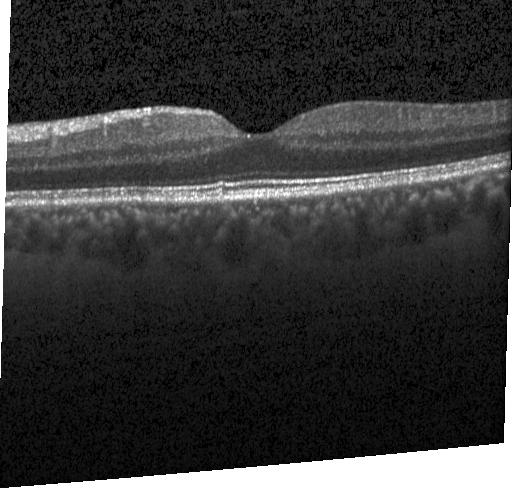 This B-scan demonstrates no evidence of choroidal neovascularization, diabetic macular edema, or drusen.